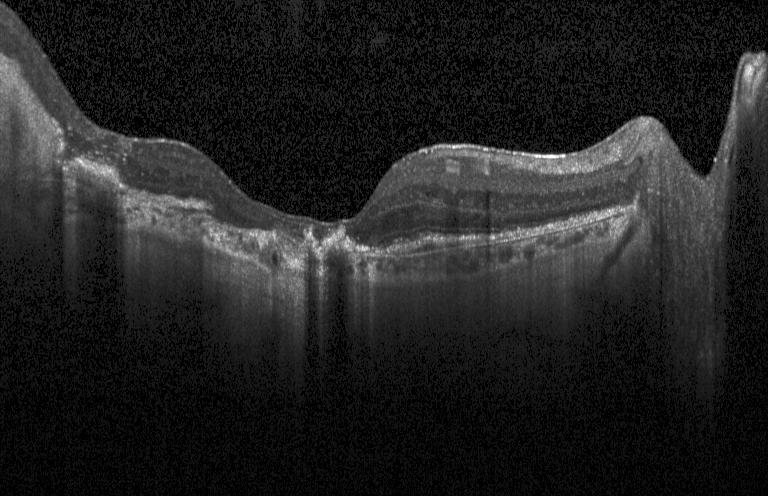 Optical coherence tomography B-scan — Finding: a choroidal neovascular membrane.